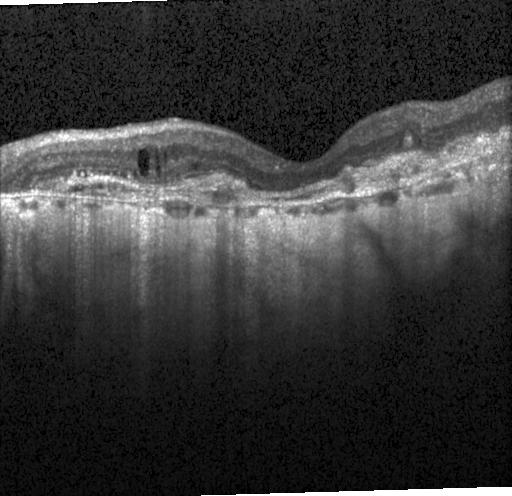 Finding: a choroidal neovascular membrane.